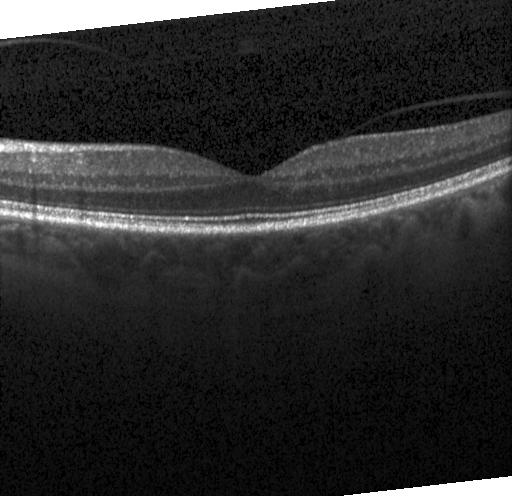 OCT finding: neither choroidal neovascularization, diabetic macular edema, nor drusen.